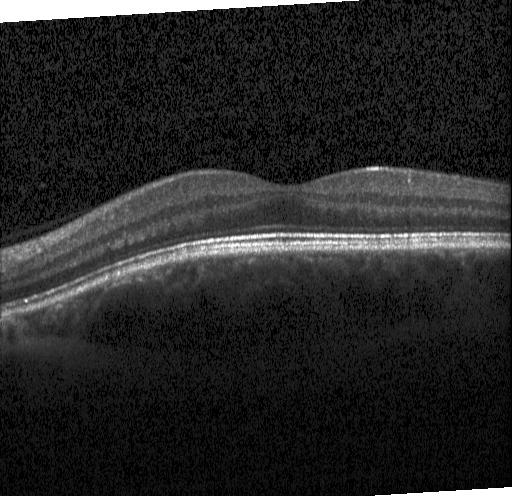
Macular OCT: neither CNV, DME, nor drusen.